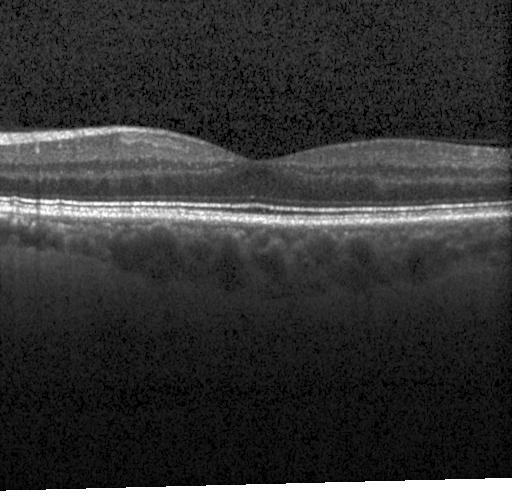
Spectral-domain OCT; through the macula; acquired on a Heidelberg Spectralis; optical coherence tomography scan — Assessment: neither choroidal neovascularization, diabetic macular edema, nor drusen.